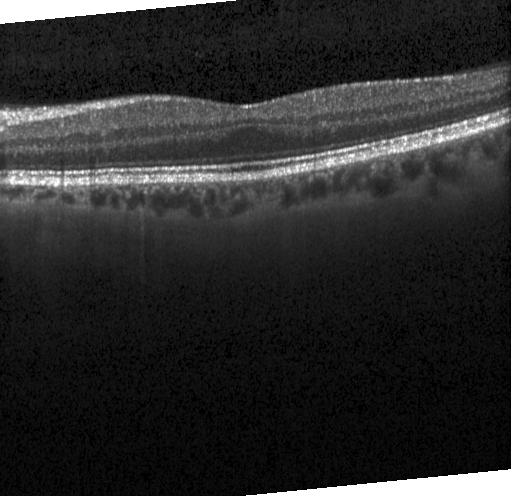

OCT line scan. Acquired on a Heidelberg Spectralis. Spectral-domain OCT — This B-scan demonstrates no evidence of choroidal neovascularization, diabetic macular edema, or drusen.